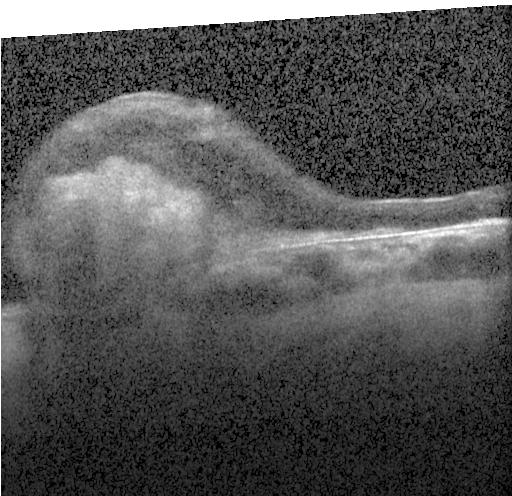 Heidelberg Spectralis OCT system. Optical coherence tomography B-scan.
Diagnosis: a choroidal neovascular membrane.